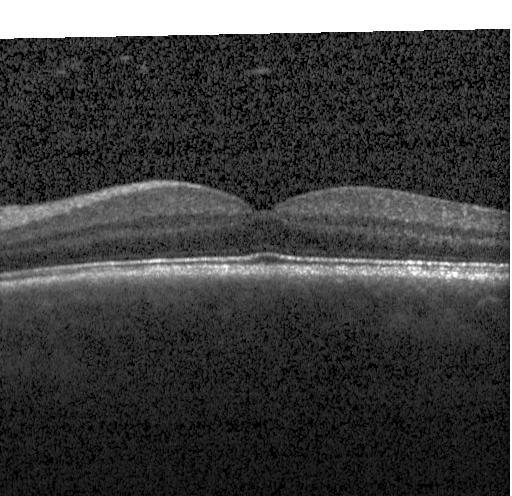

Finding: no CNV, no DME, and no drusen.